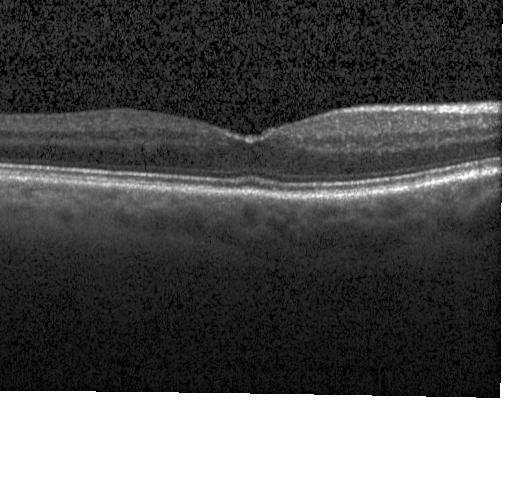

Acquired on a Heidelberg Spectralis; horizontal scan through the fovea; OCT line scan; SD-OCT.
Assessment: no choroidal neovascularization, diabetic macular edema, or drusen.